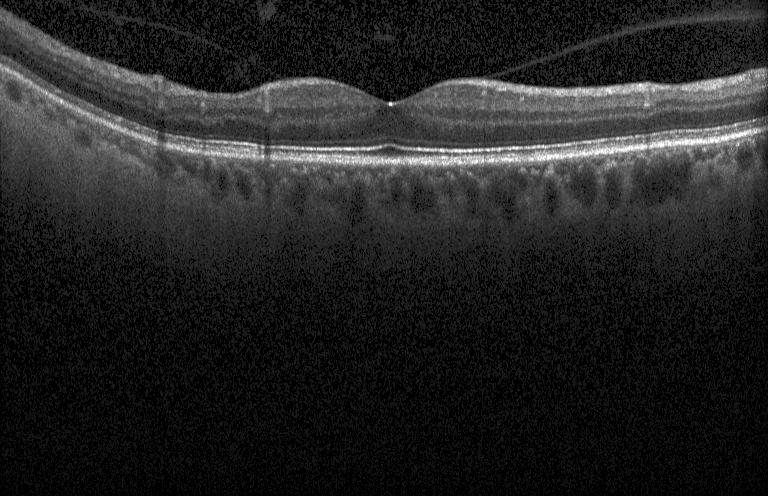

Impression: no choroidal neovascularization, no diabetic macular edema, and no drusen.